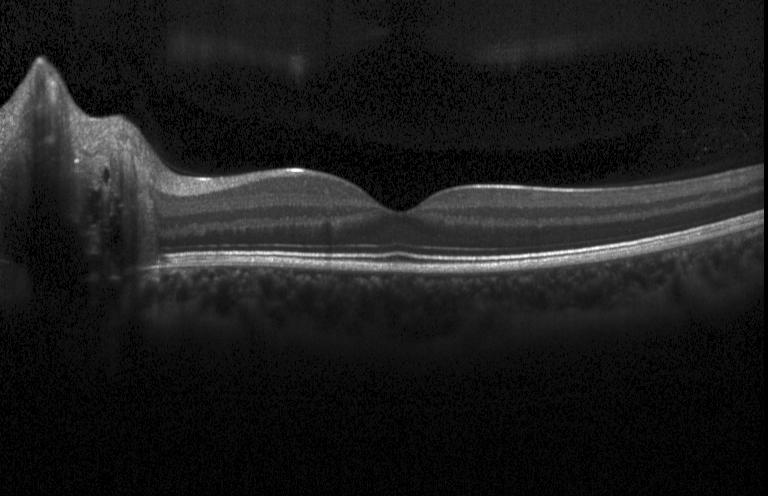

Macular OCT: no CNV, DME, or drusen.